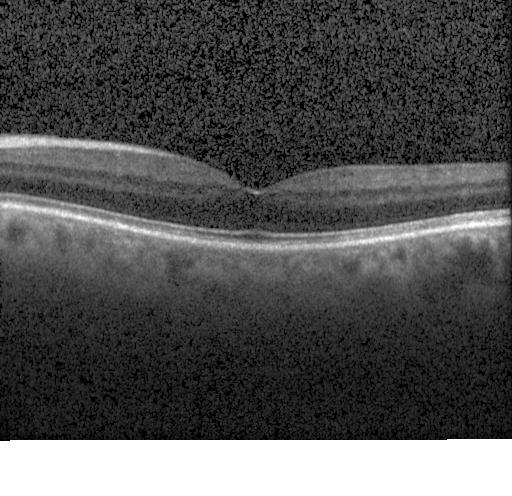

This B-scan demonstrates no choroidal neovascularization, no diabetic macular edema, and no drusen.